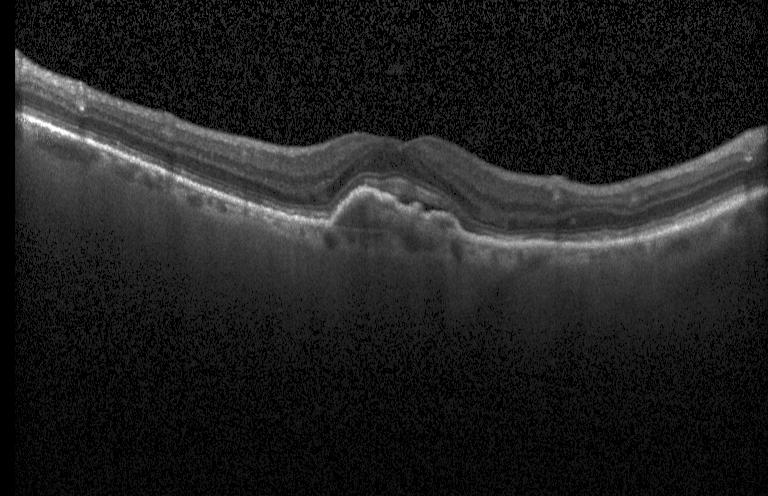

OCT finding: a choroidal neovascular membrane.